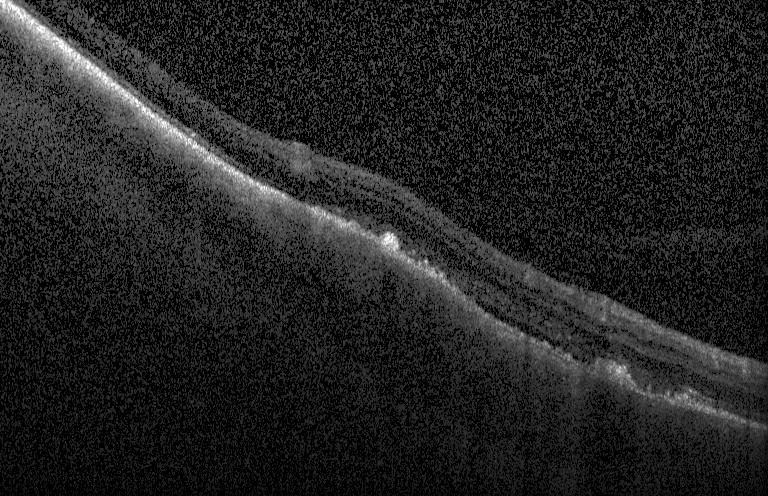

Optical coherence tomography scan
Impression: CNV.